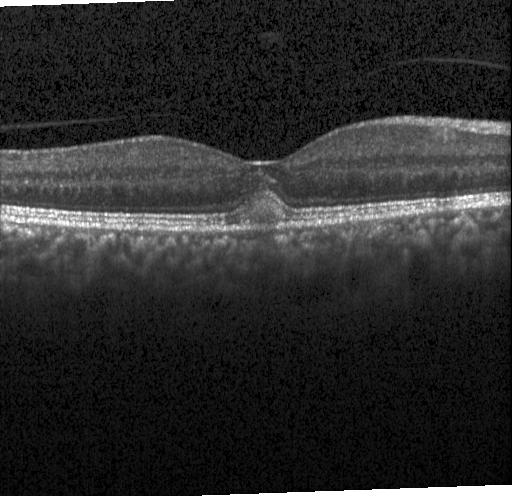

Heidelberg Spectralis; retinal OCT cross-section; SD-OCT
Impression: a choroidal neovascular membrane.